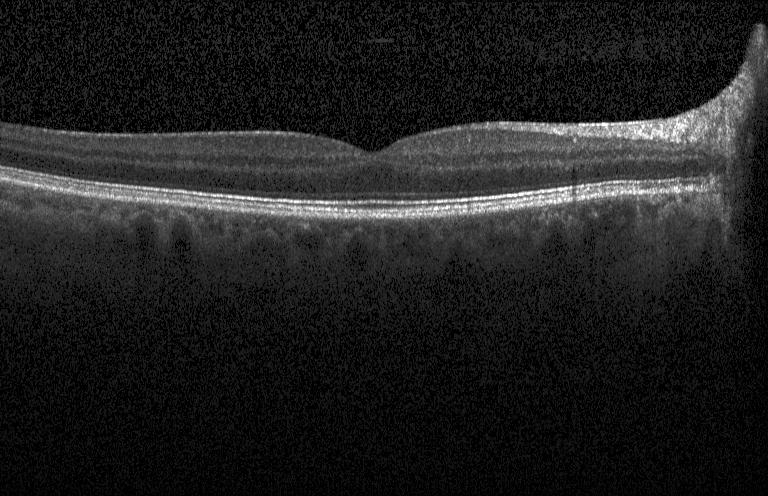
Retinal OCT cross-section showing neither choroidal neovascularization, diabetic macular edema, nor drusen.